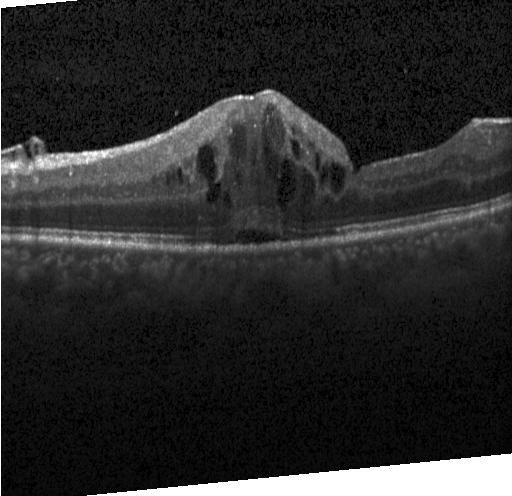
Finding: diabetic macular edema.